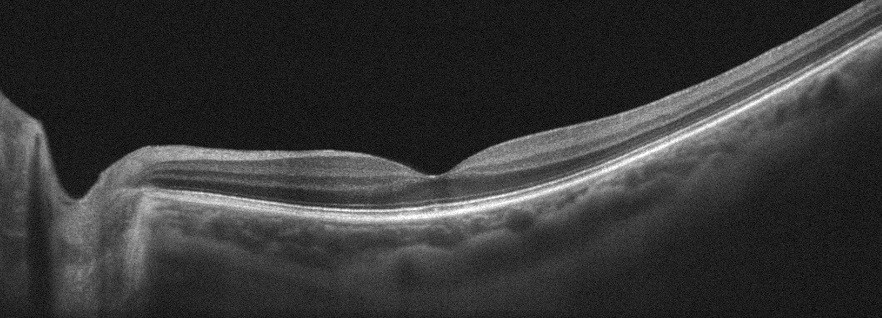
OCT line scan.
Dx: no AMD, DME, ERM, RAO, RVO, or VID.